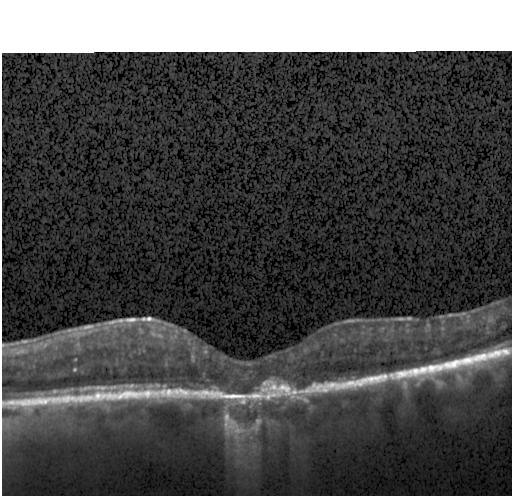
This B-scan demonstrates a choroidal neovascular membrane.